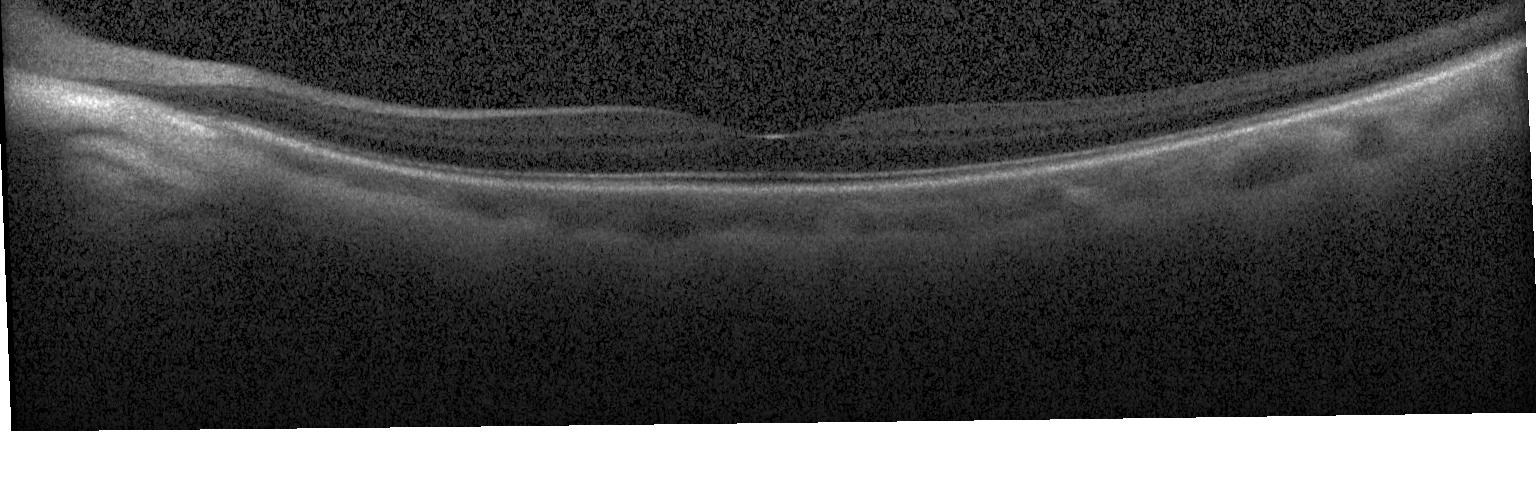 Spectral-domain OCT. OCT line scan
Impression: no CNV, DME, or drusen.